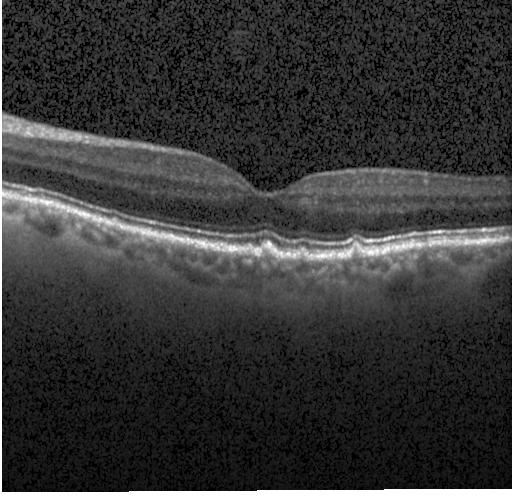
OCT finding: multiple drusen.